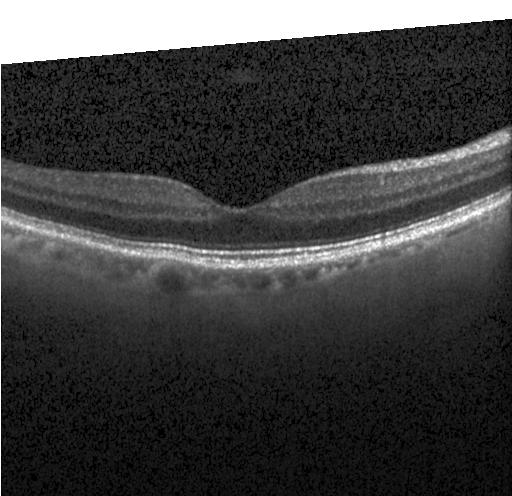 Spectral-domain optical coherence tomography · retinal OCT cross-section · Heidelberg Spectralis. Assessment: no choroidal neovascularization, no diabetic macular edema, and no drusen.